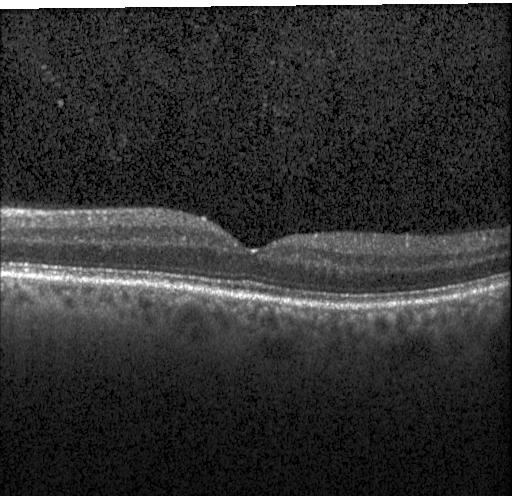 Retinal OCT cross-section — OCT finding: no CNV, DME, or drusen.